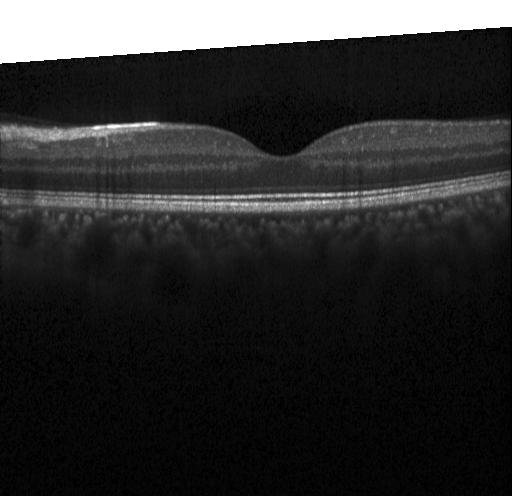 Heidelberg Spectralis OCT system, horizontal scan through the fovea, retinal OCT cross-section, spectral-domain optical coherence tomography — Impression: no CNV, no DME, and no drusen.